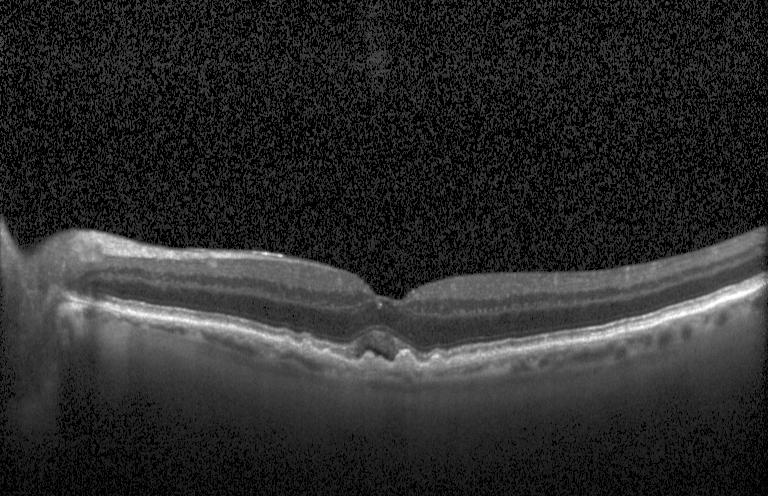

Optical coherence tomography scan, spectral-domain optical coherence tomography, Heidelberg Spectralis OCT system, horizontal scan through the fovea. Impression: choroidal neovascularization (CNV).